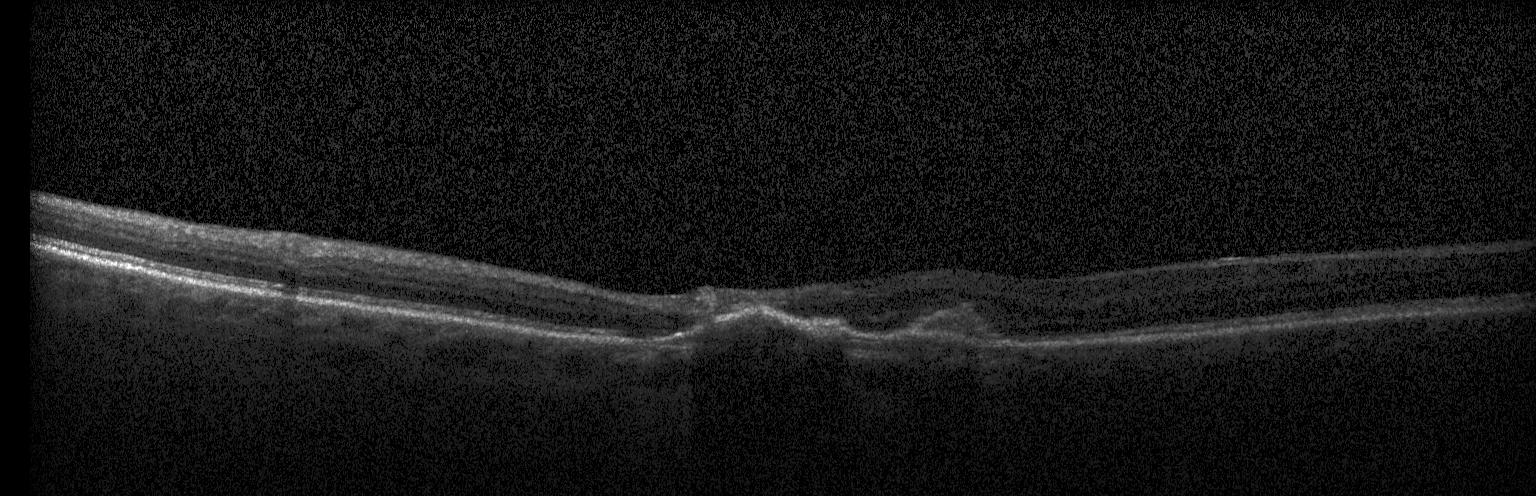 This B-scan demonstrates a choroidal neovascular membrane.